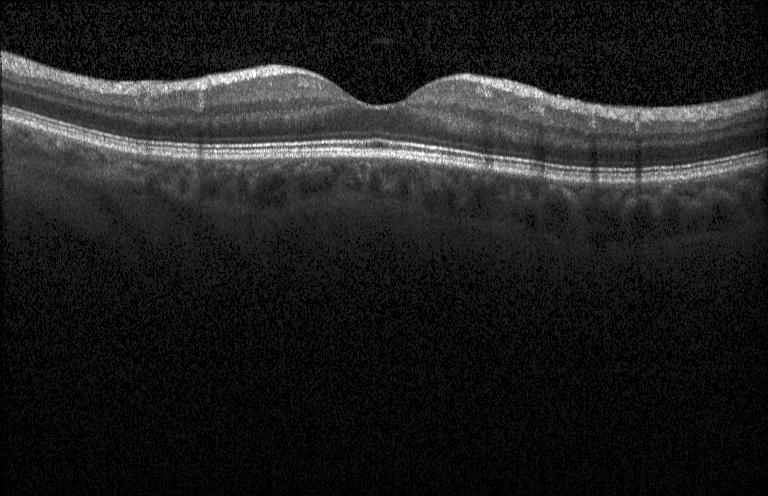
Retinal OCT cross-section showing neither choroidal neovascularization, diabetic macular edema, nor drusen.